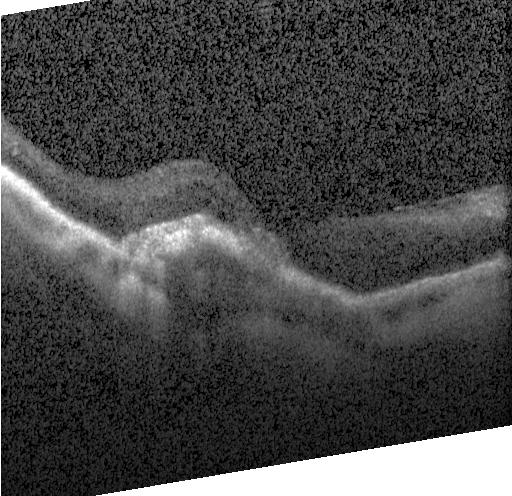
Retinal OCT cross-section. Fovea-centered. Heidelberg Spectralis
Assessment: CNV.